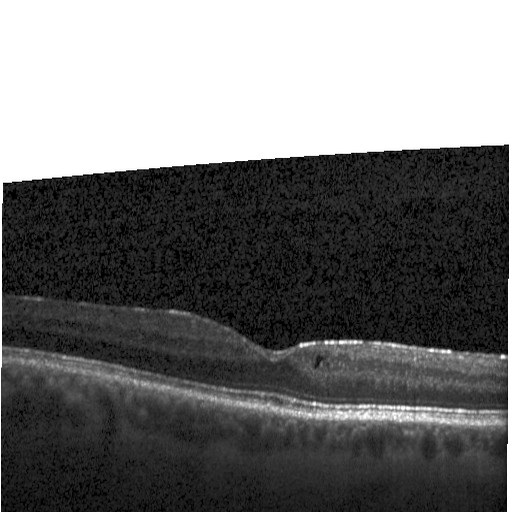

Macular scan. Heidelberg Spectralis OCT system. Retinal OCT B-scan. SD-OCT
The scan shows diabetic macular edema (DME).